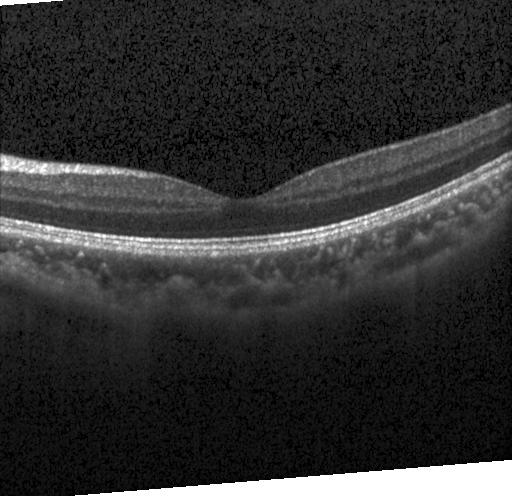
Horizontal scan through the fovea, instrument: Heidelberg Spectralis, optical coherence tomography B-scan.
Dx: no choroidal neovascularization, diabetic macular edema, or drusen.